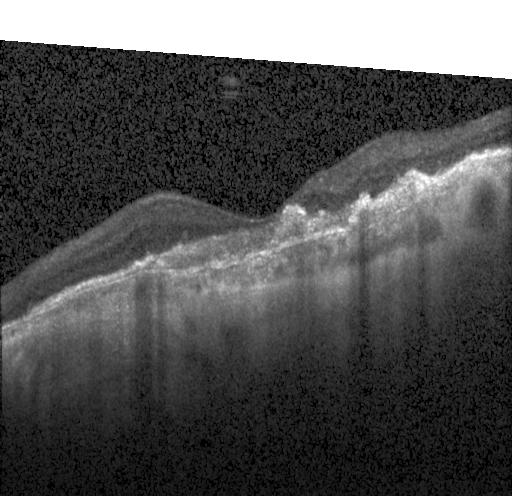
Optical coherence tomography scan — Assessment: a choroidal neovascular membrane.